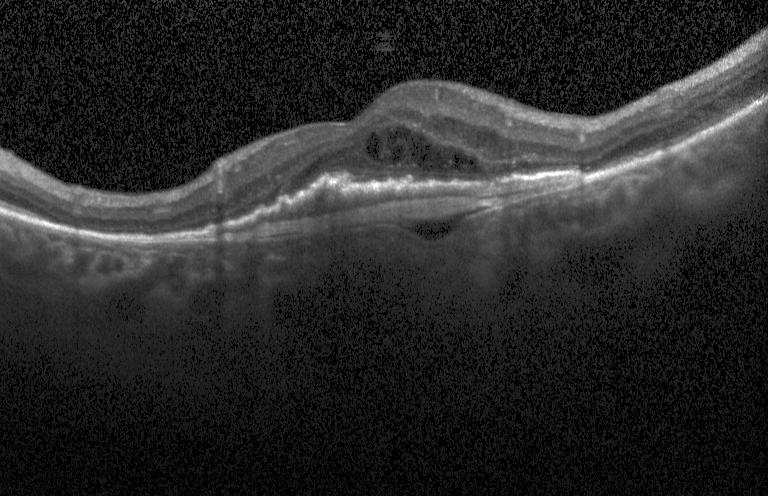 OCT line scan. Centered on the fovea.
The scan shows a choroidal neovascular membrane.